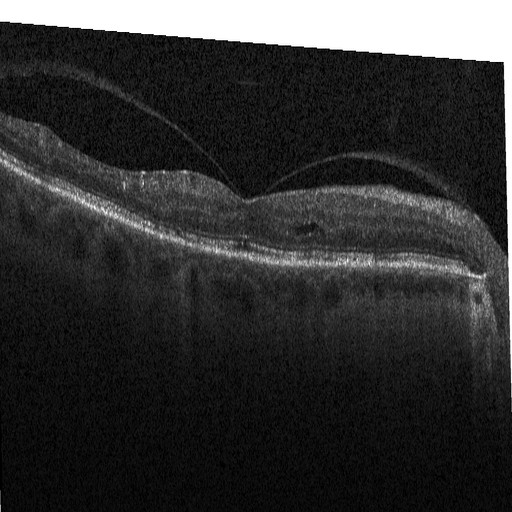 Impression: diabetic macular edema (DME).